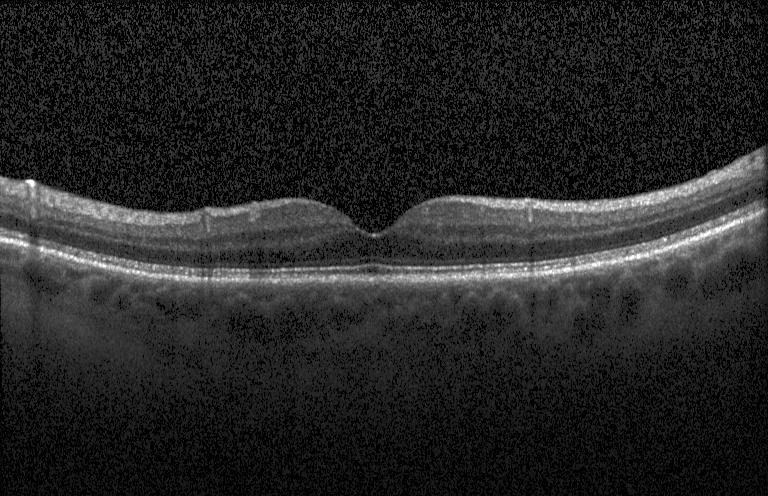 OCT line scan · spectral-domain OCT · macular scan · Heidelberg Spectralis. Finding: no choroidal neovascularization, no diabetic macular edema, and no drusen.